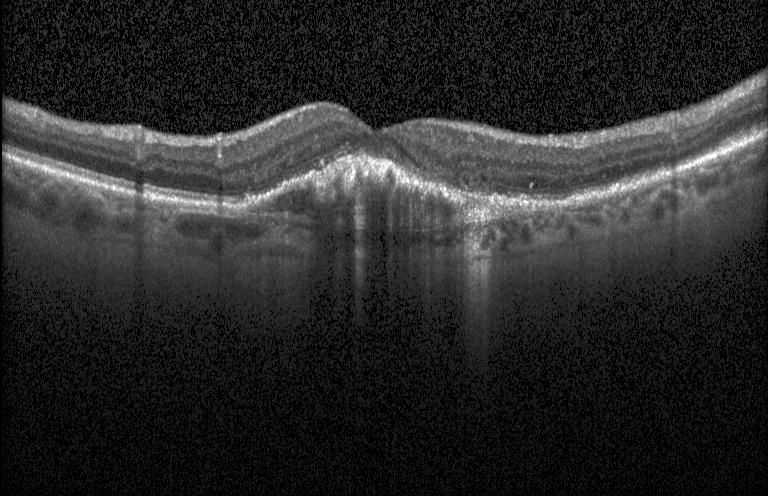 Choroidal neovascularization (CNV).